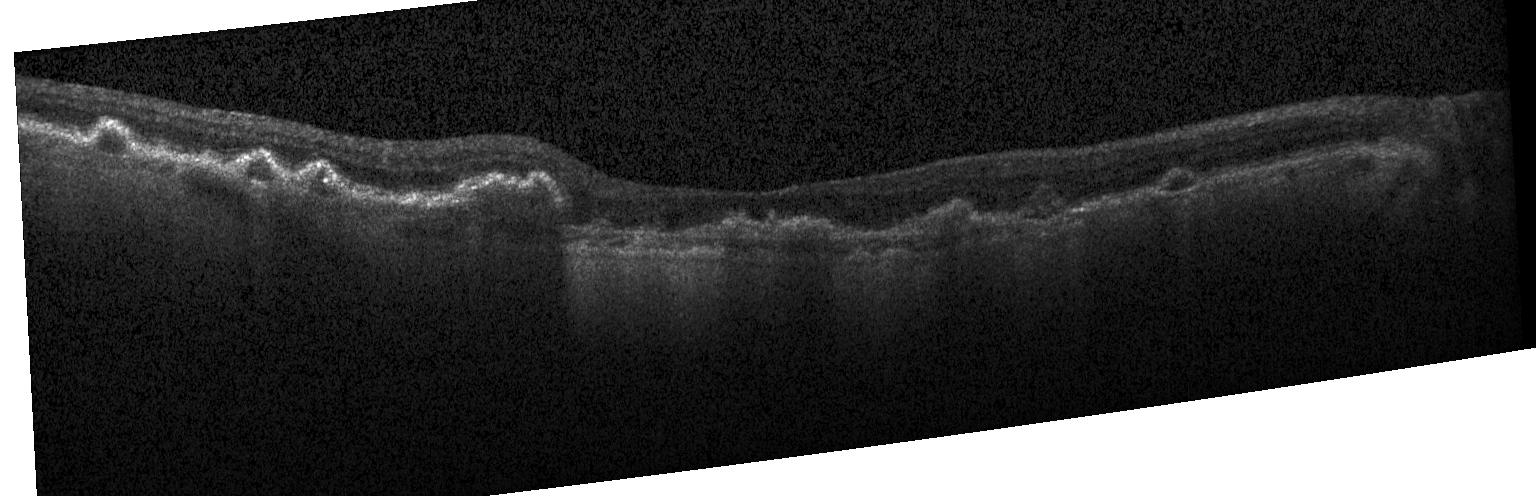
Finding: CNV.